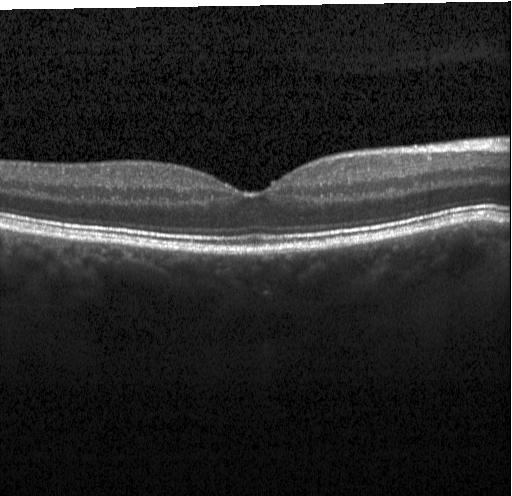

Retinal OCT B-scan — Assessment: no choroidal neovascularization, no diabetic macular edema, and no drusen.